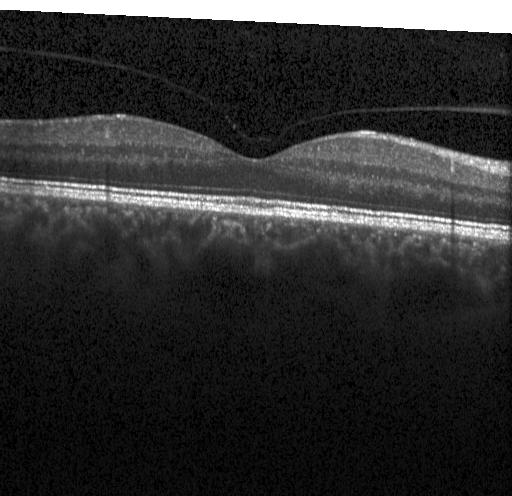

Optical coherence tomography scan · instrument: Heidelberg Spectralis · SD-OCT · macular scan. Dx: no choroidal neovascularization, diabetic macular edema, or drusen.